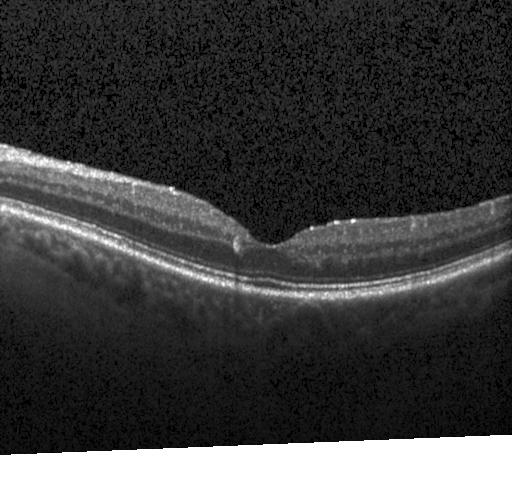

OCT scan showing no evidence of choroidal neovascularization, diabetic macular edema, or drusen.